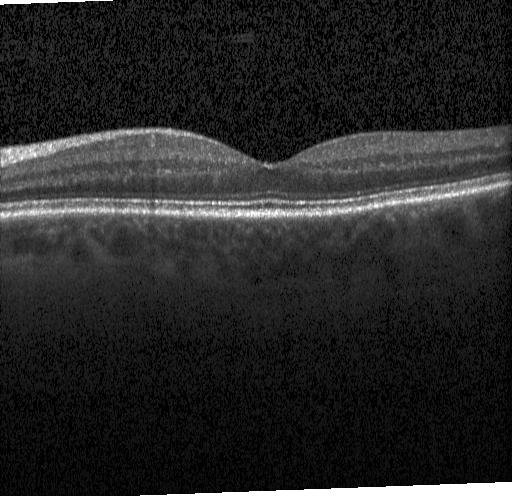 Optical coherence tomography scan; horizontal scan through the fovea. Impression: neither CNV, DME, nor drusen.